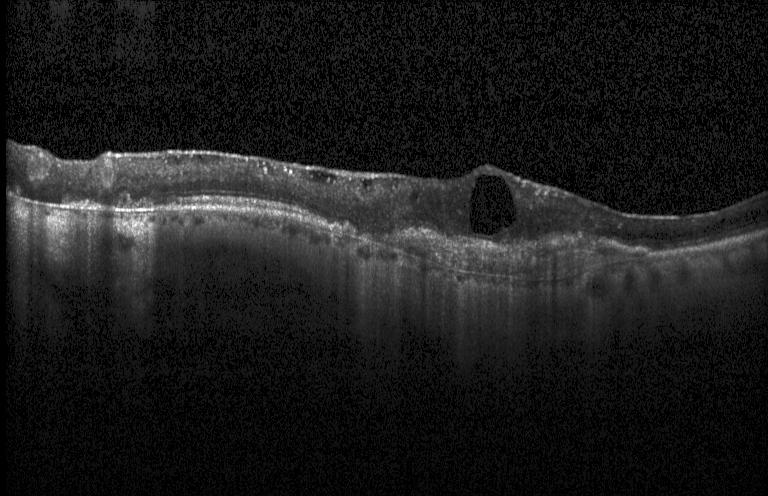
Diagnosis: choroidal neovascularization (CNV).